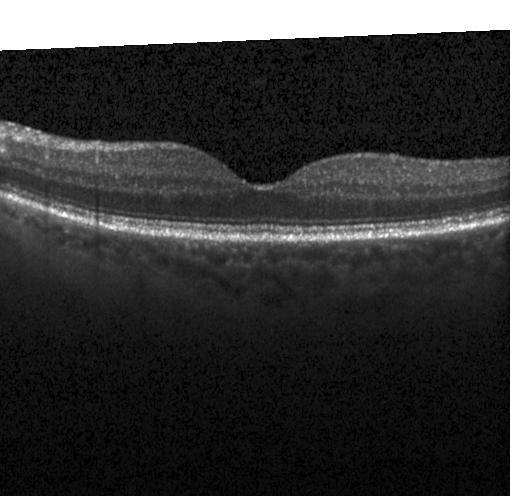

Spectral-domain OCT, OCT B-scan. The scan shows no choroidal neovascularization, diabetic macular edema, or drusen.